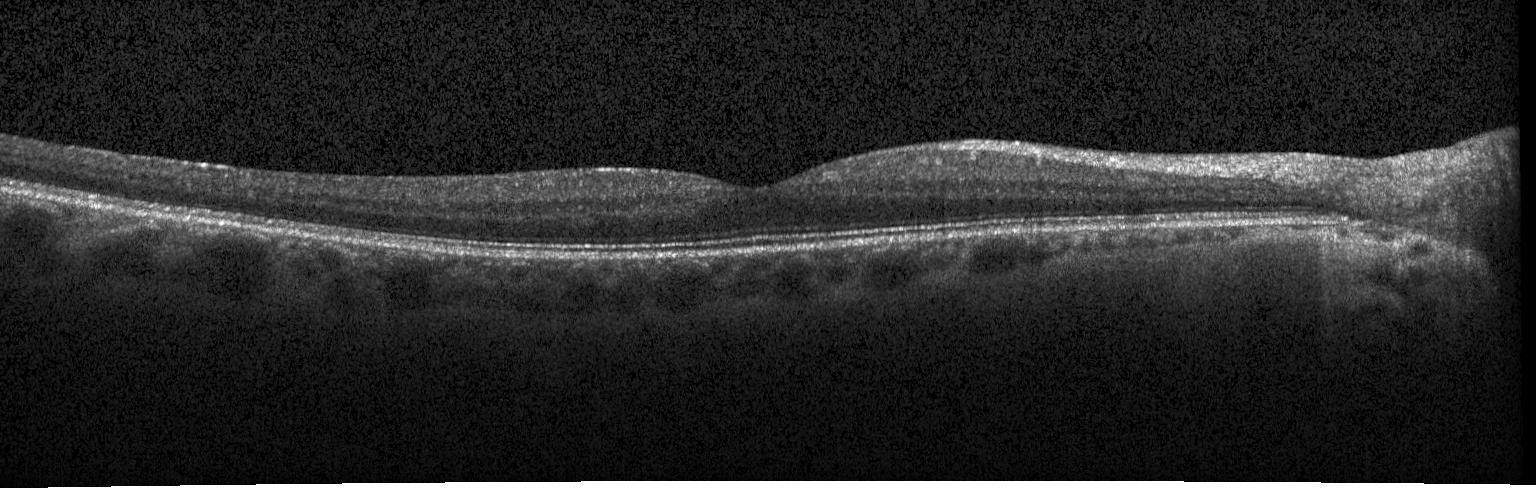 Dx: no CNV, no DME, and no drusen.